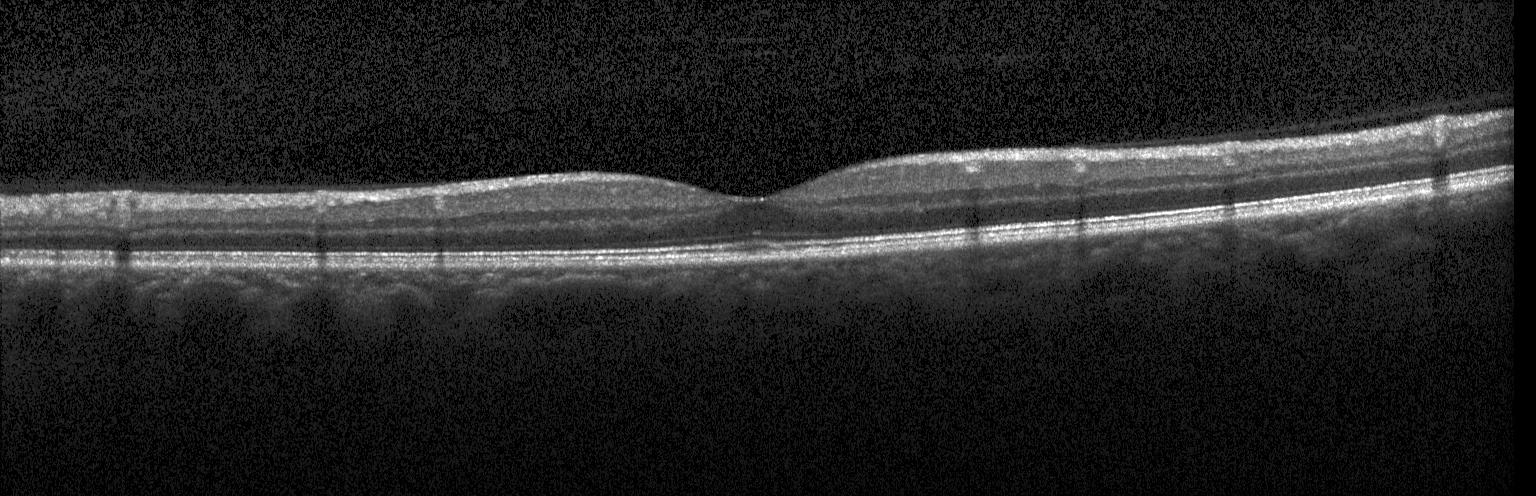

Finding: neither CNV, DME, nor drusen.